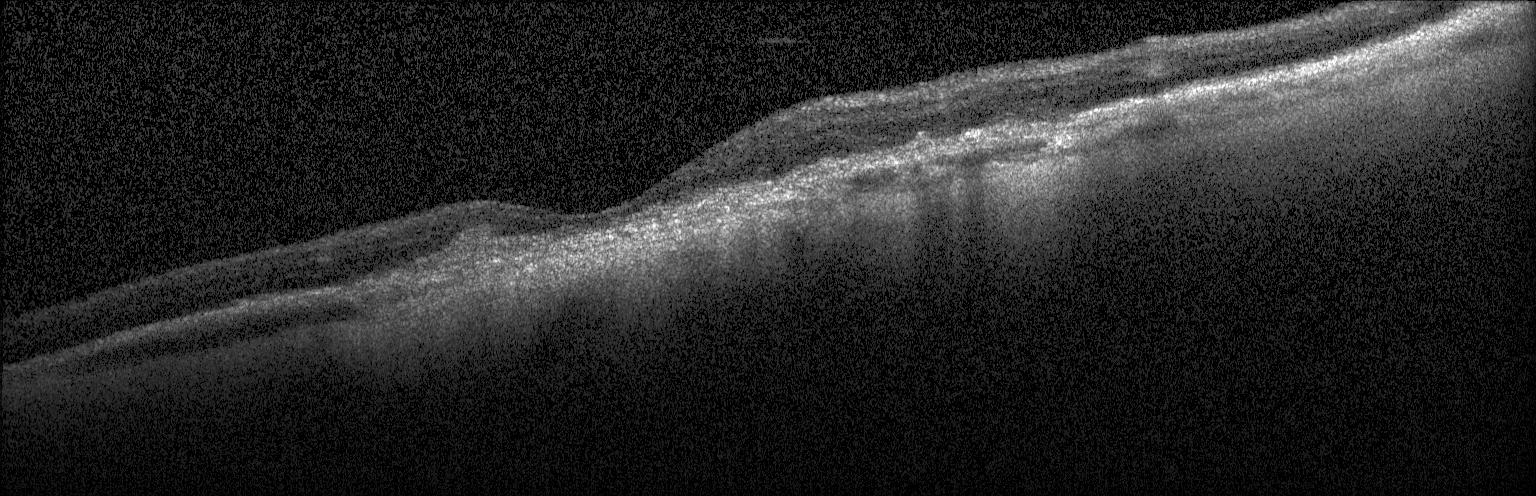
Spectral-domain OCT · retinal OCT cross-section
Impression: a choroidal neovascular membrane.